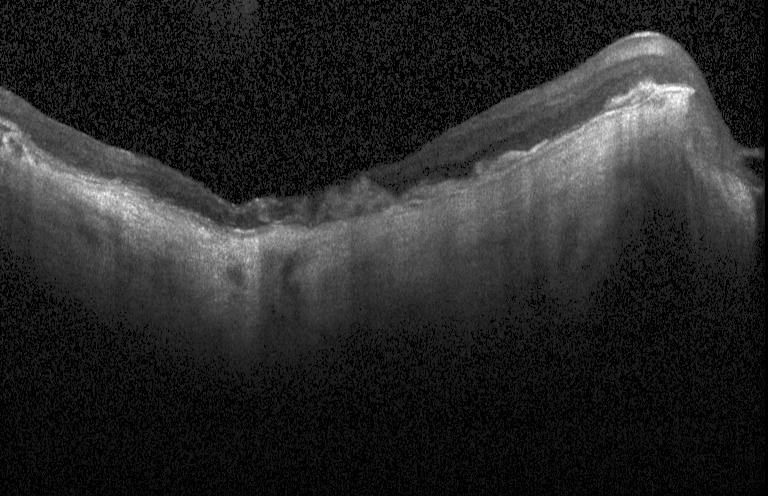
Spectral-domain optical coherence tomography. Fovea-centered. Optical coherence tomography scan. Instrument: Heidelberg Spectralis. Impression: choroidal neovascularization.